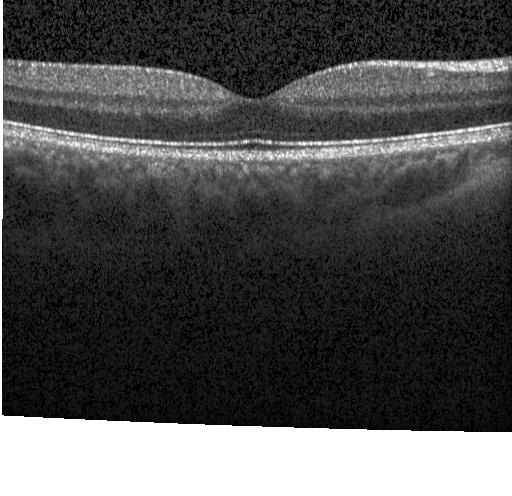
OCT finding: no choroidal neovascularization, no diabetic macular edema, and no drusen.